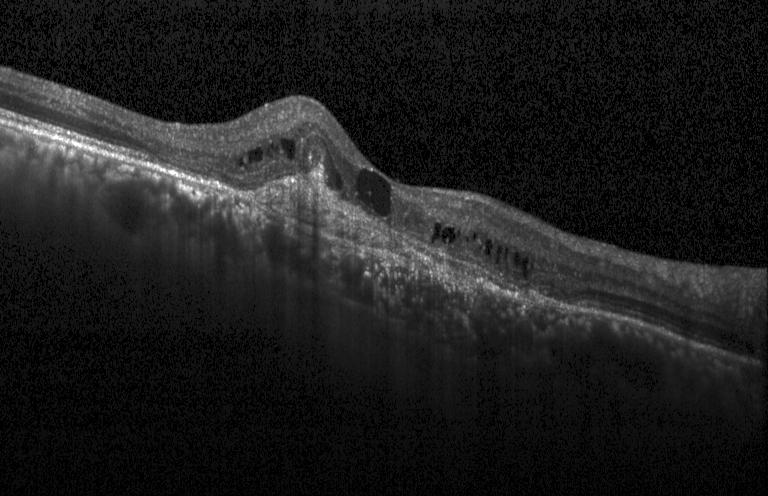 Diagnosis: choroidal neovascularization (CNV).